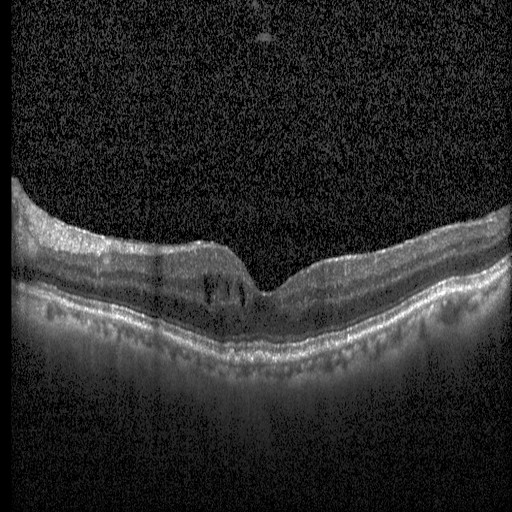
This B-scan demonstrates DME.